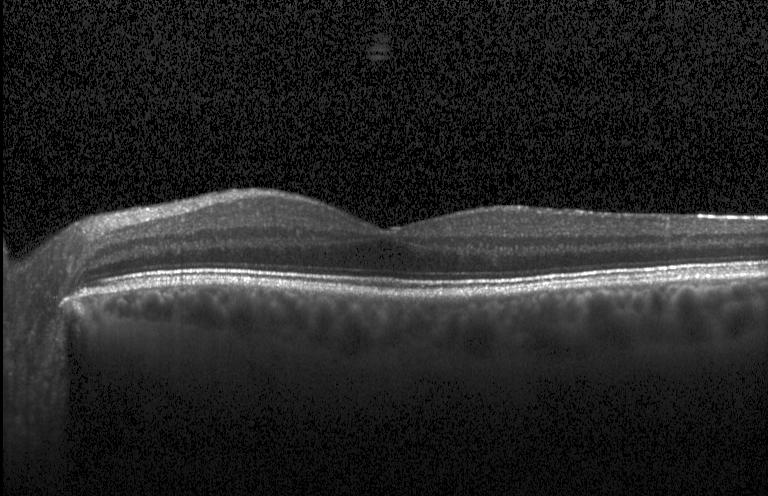
Macular OCT demonstrating neither choroidal neovascularization, diabetic macular edema, nor drusen.